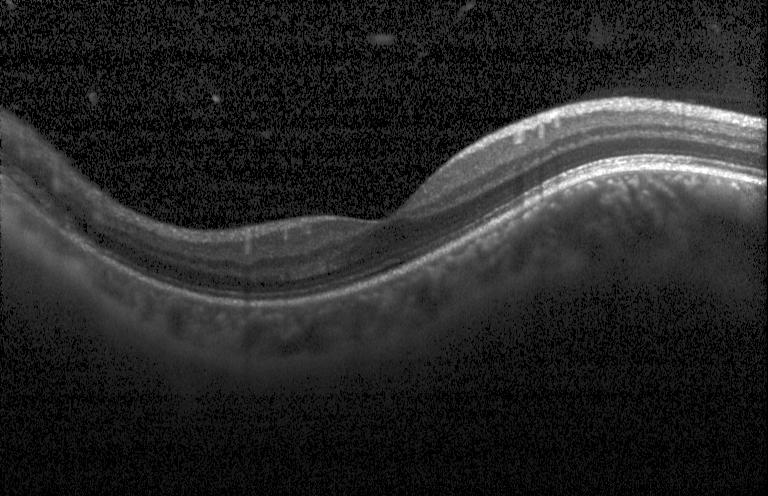

Impression: no evidence of CNV, DME, or drusen.